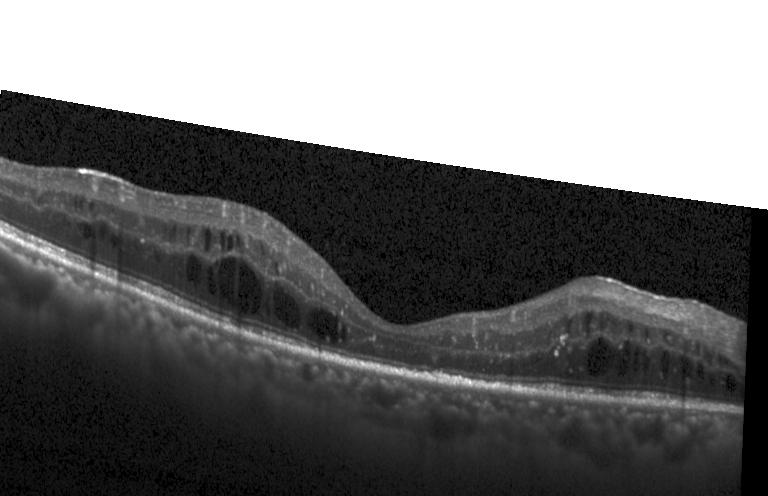

Heidelberg Spectralis; retinal OCT B-scan.
Diagnosis: diabetic macular edema (DME).